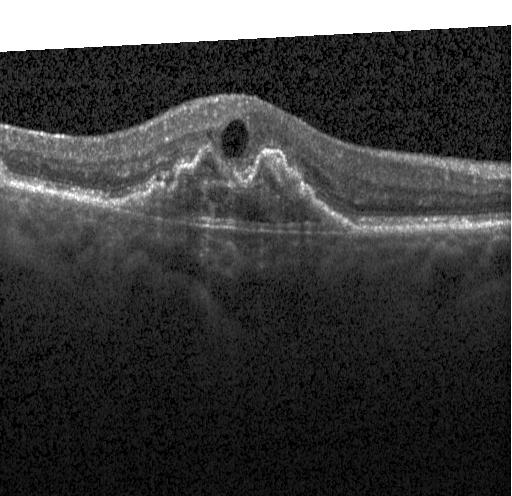
Retinal OCT cross-section · instrument: Heidelberg Spectralis — Impression: CNV.